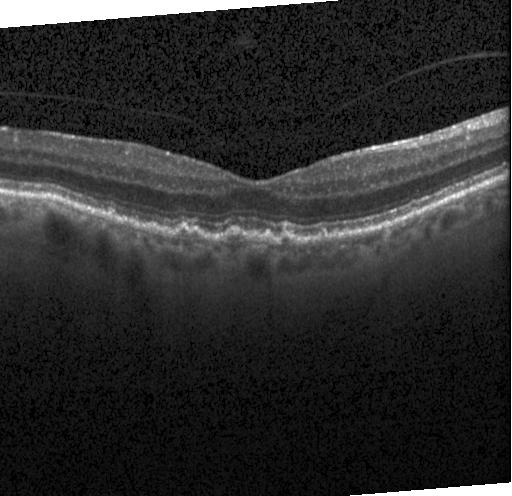

OCT B-scan, horizontal scan through the fovea. Impression: multiple drusen.